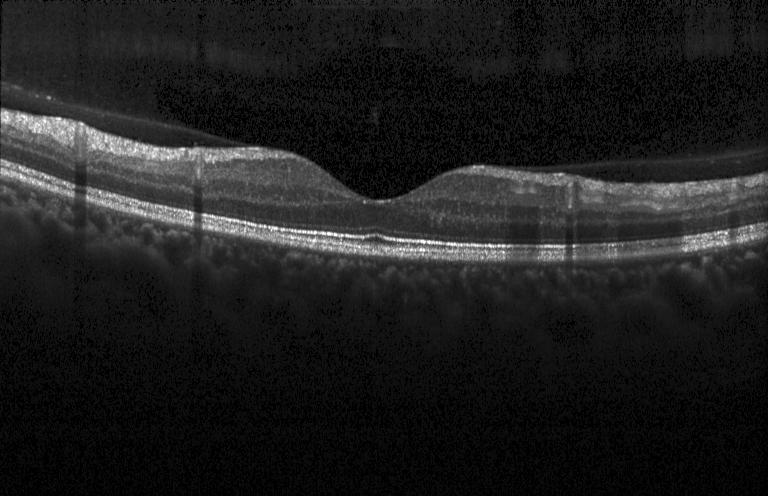 Impression: no CNV, no DME, and no drusen.